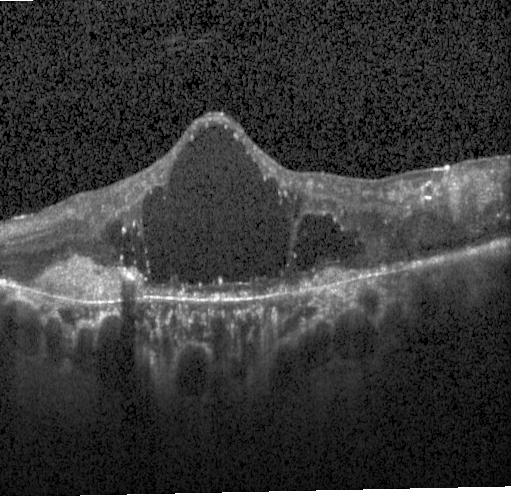 OCT line scan. This B-scan demonstrates choroidal neovascularization (CNV).